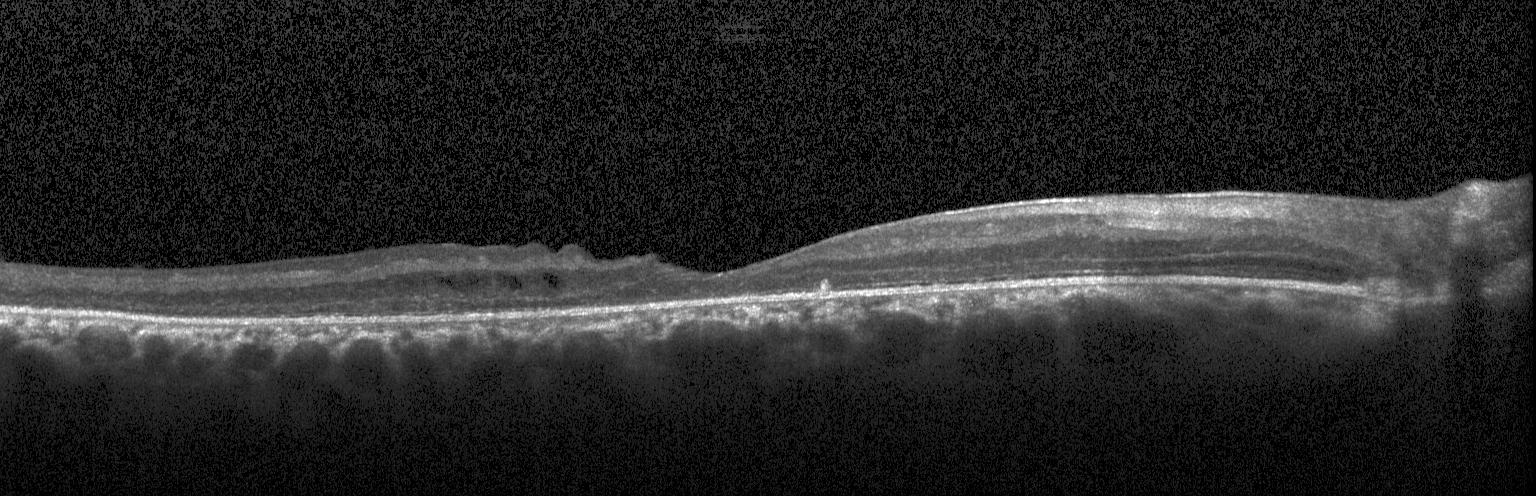

Heidelberg Spectralis, retinal OCT B-scan — Diagnosis: diabetic macular edema (DME).